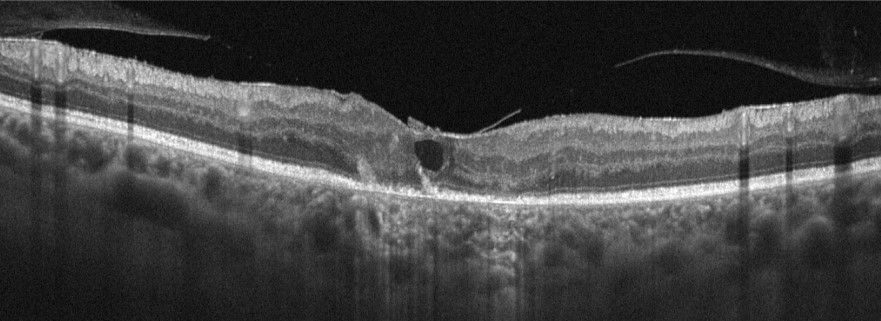 OCT B-scan, through the macula.
This B-scan demonstrates DME.